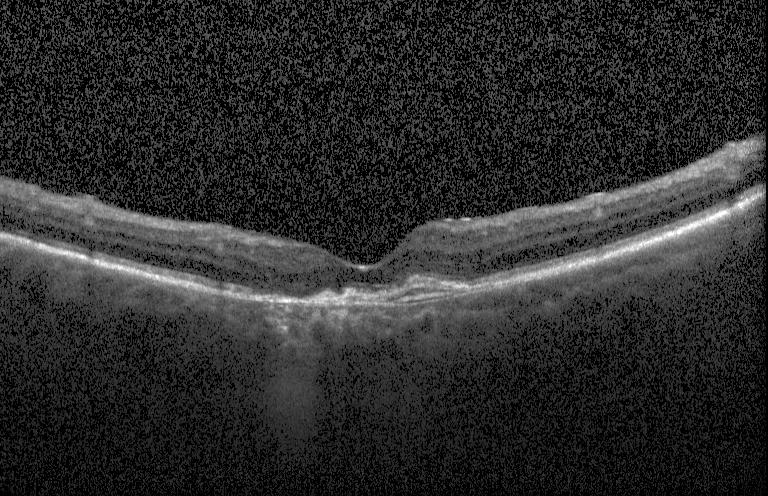 Assessment: CNV.